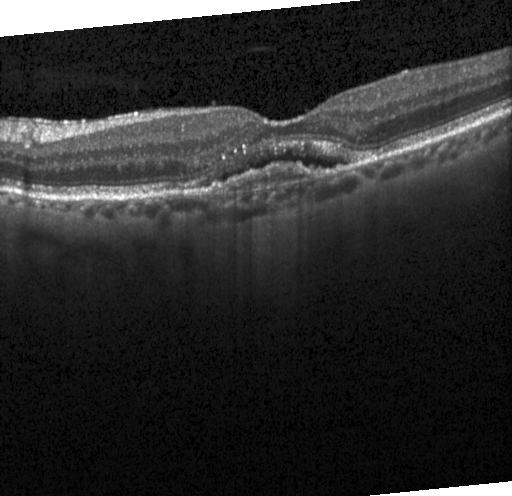
Instrument: Heidelberg Spectralis · optical coherence tomography scan
The scan shows a choroidal neovascular membrane.